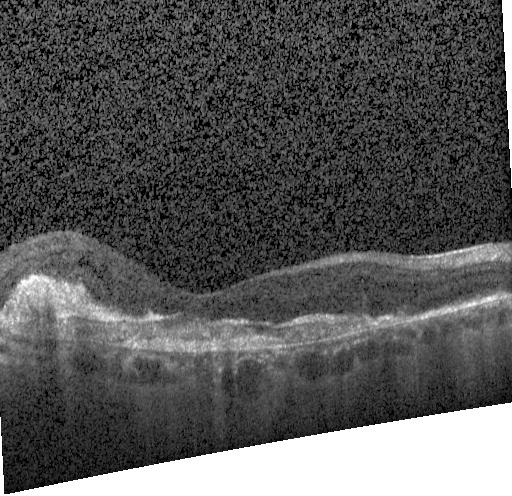
Centered on the fovea · OCT line scan.
Impression: a choroidal neovascular membrane.